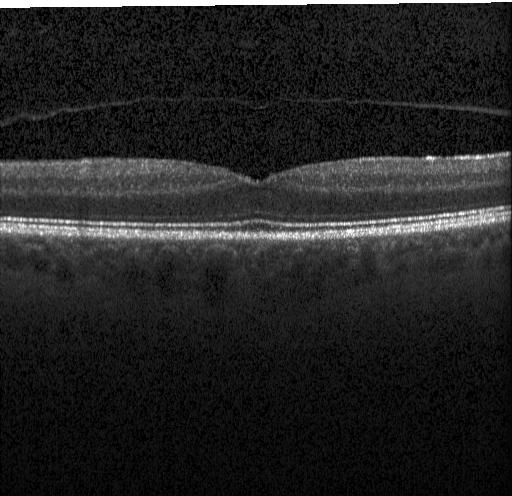 Finding: no choroidal neovascularization, diabetic macular edema, or drusen.